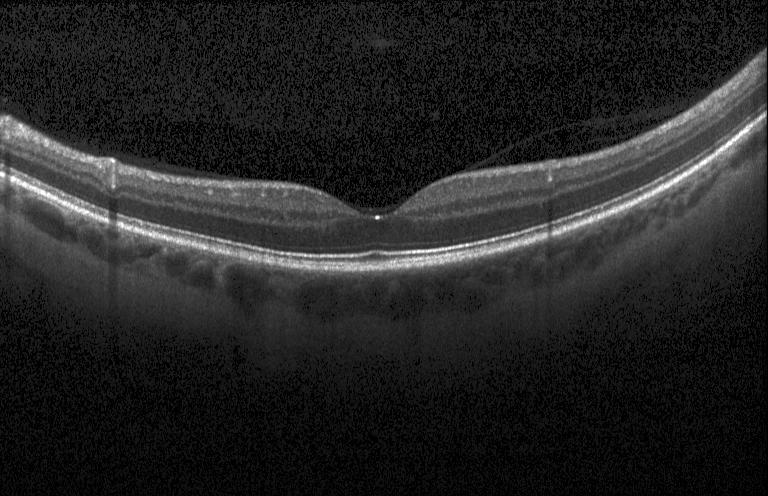

Retinal OCT cross-section showing no CNV, no DME, and no drusen.